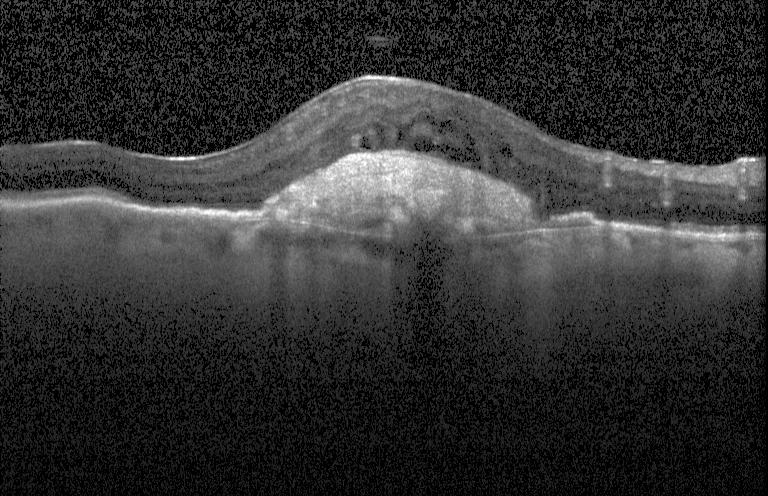
Retinal OCT cross-section
Diagnosis: a choroidal neovascular membrane.